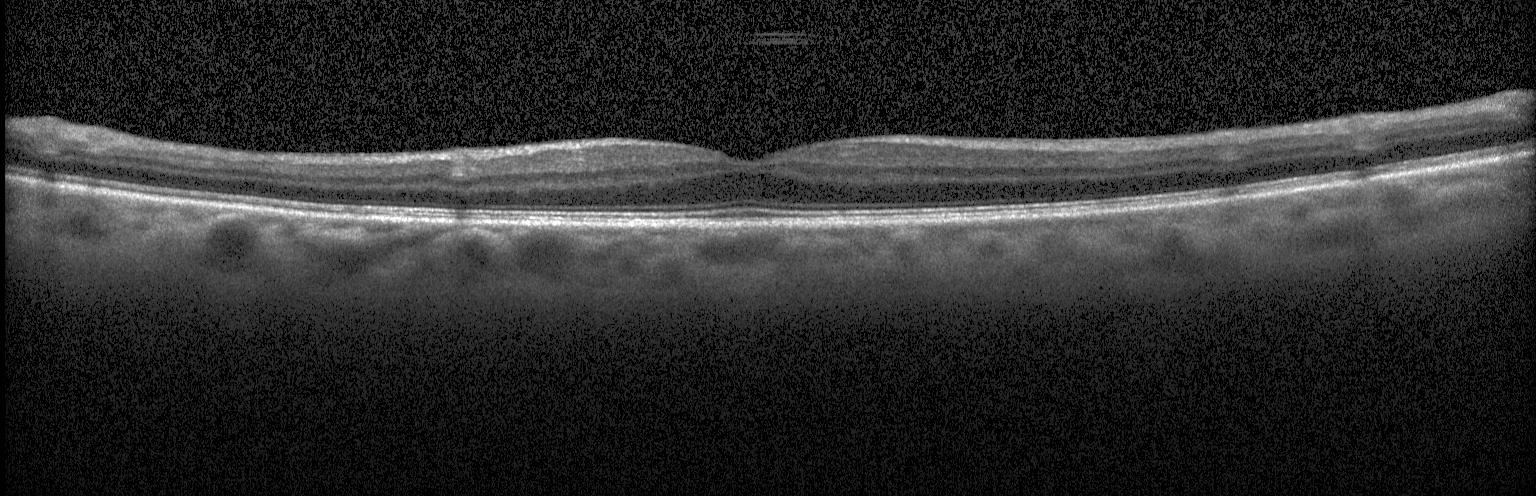
Macular OCT: no evidence of CNV, DME, or drusen.